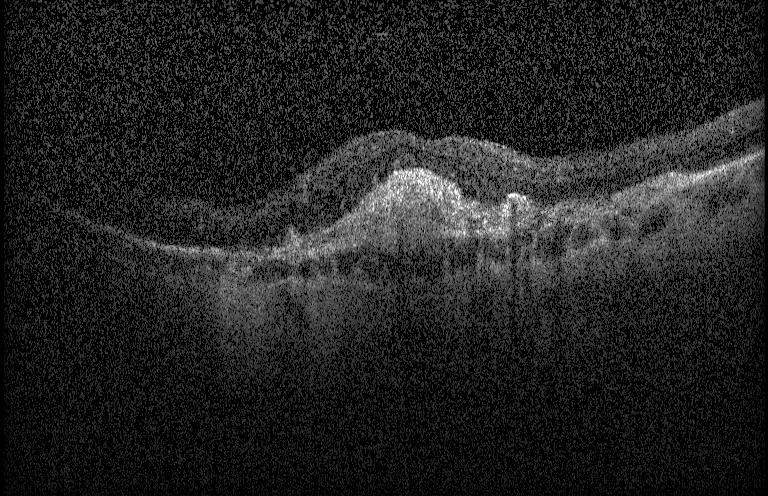

Macular OCT: CNV.